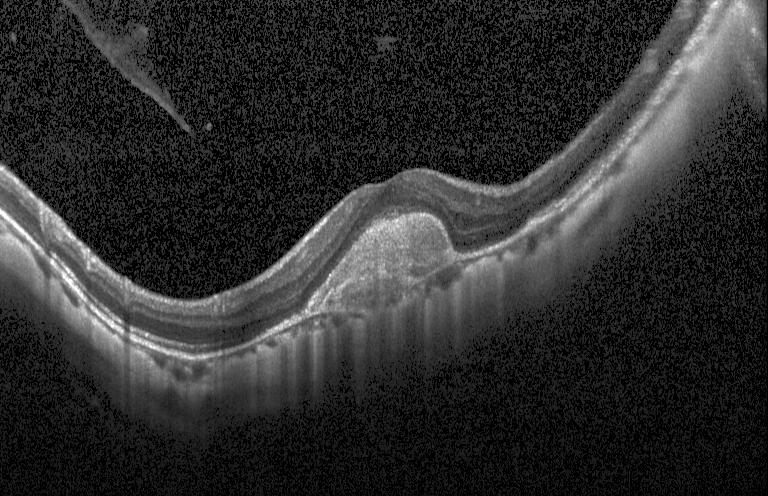
Retinal OCT cross-section. Finding: choroidal neovascularization (CNV).